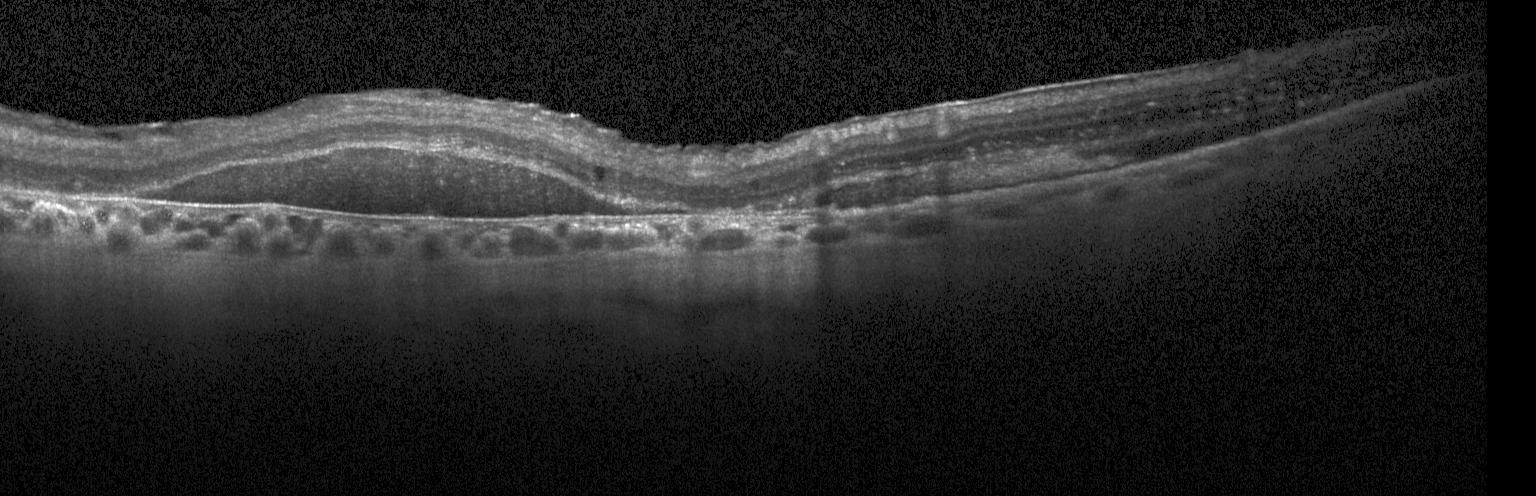
Retinal OCT B-scan; spectral-domain OCT; macular scan; Heidelberg Spectralis OCT system.
Impression: a choroidal neovascular membrane.